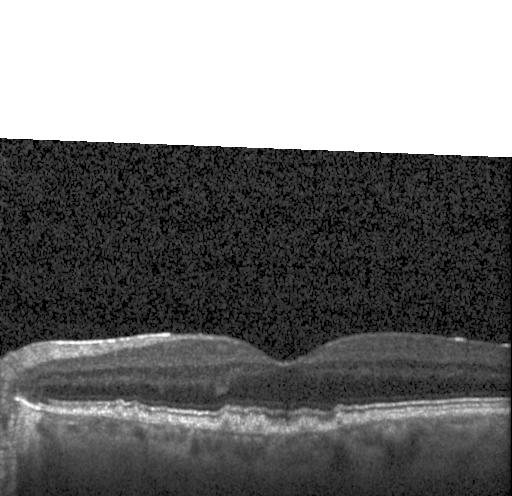
OCT scan showing multiple drusen.